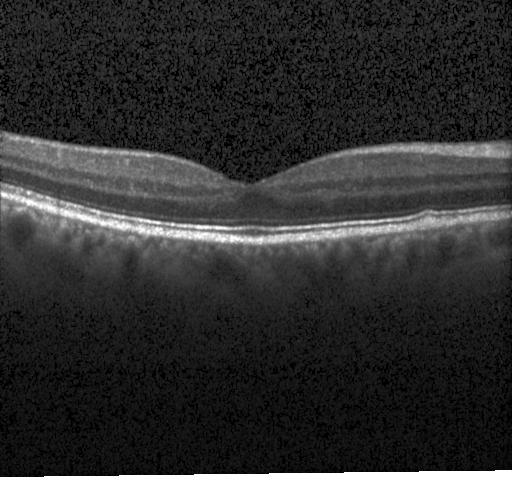
Spectral-domain OCT B-scan: sub-RPE drusenoid deposits.